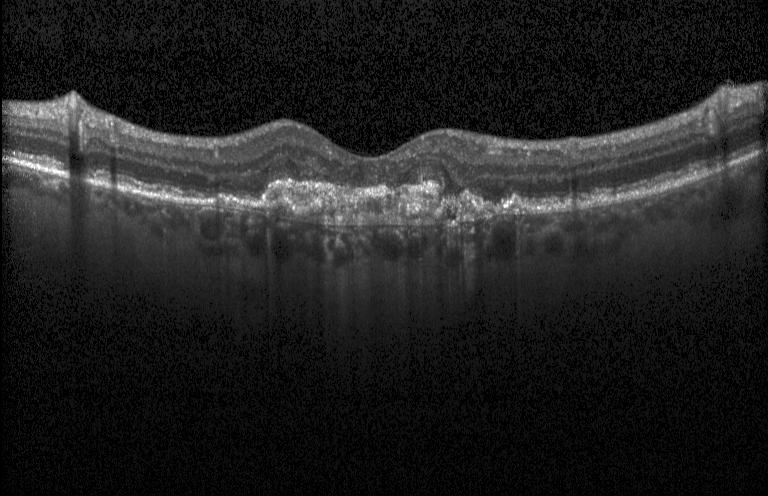

SD-OCT · fovea-centered · retinal OCT B-scan · Heidelberg Spectralis OCT system — A choroidal neovascular membrane.